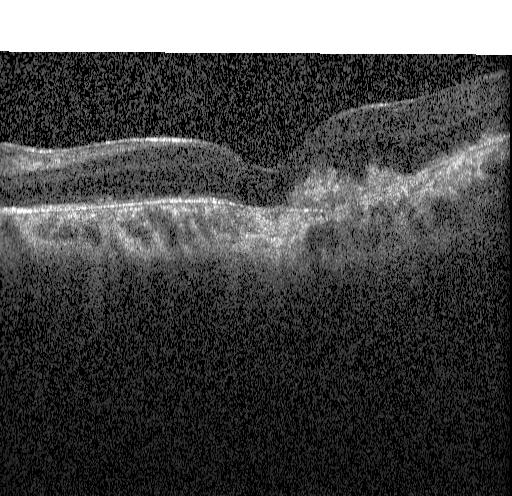 Impression: choroidal neovascularization.